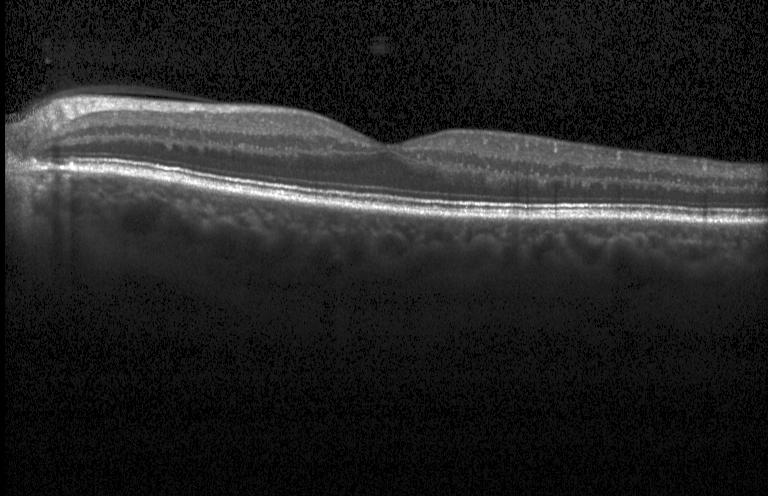
Impression: no evidence of CNV, DME, or drusen.